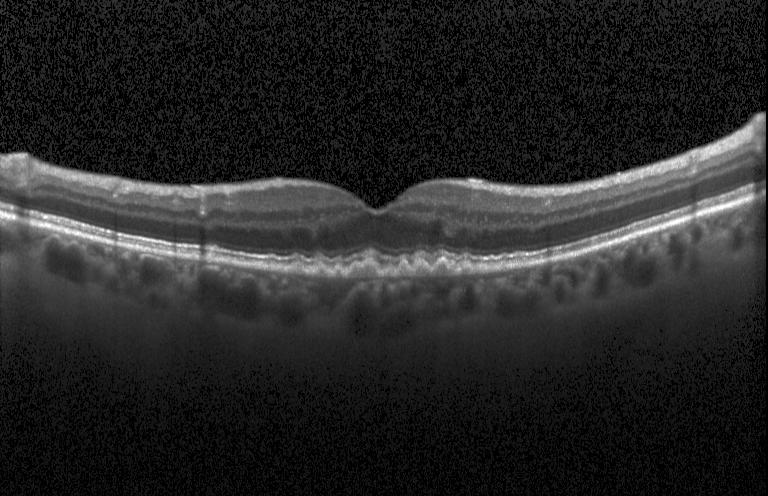 Heidelberg Spectralis OCT system; spectral-domain optical coherence tomography; OCT line scan — Impression: multiple drusen.